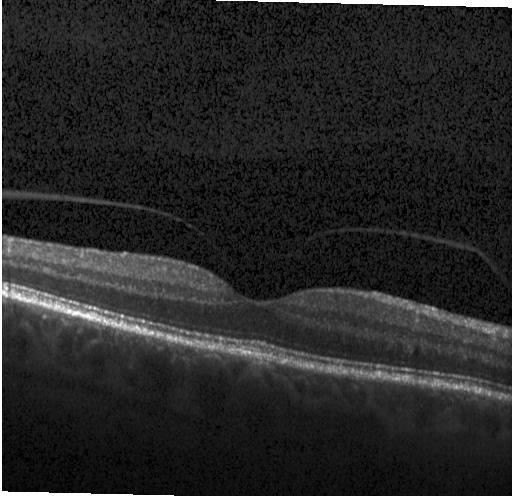 Finding: no evidence of choroidal neovascularization, diabetic macular edema, or drusen.